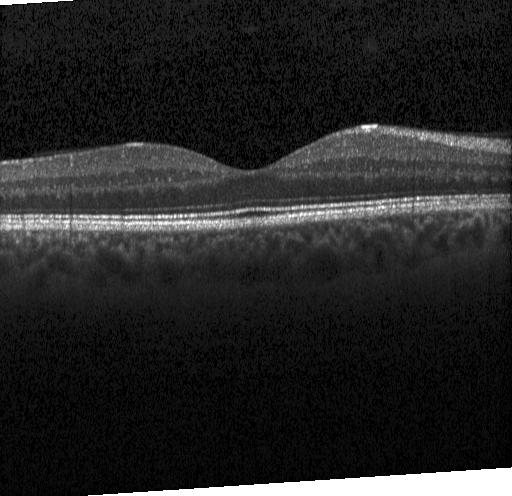 Dx: no choroidal neovascularization, no diabetic macular edema, and no drusen.